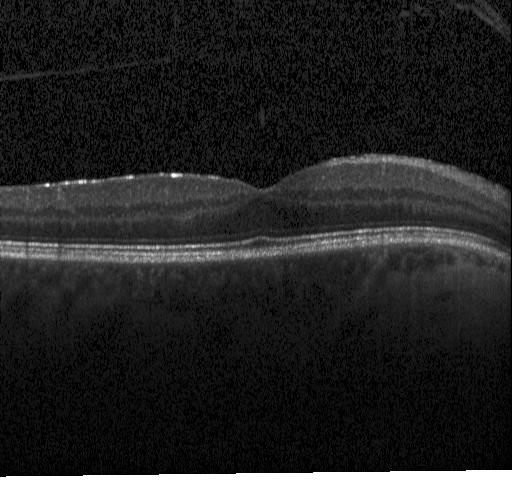 Diagnosis: no CNV, no DME, and no drusen.